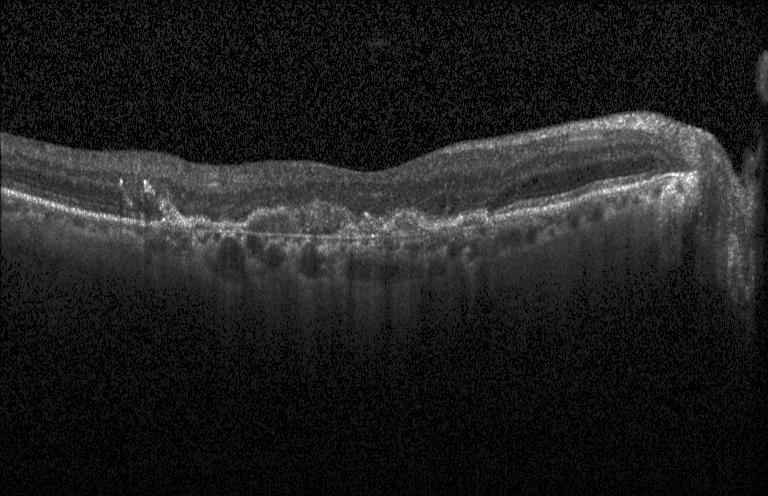 This B-scan demonstrates choroidal neovascularization (CNV).